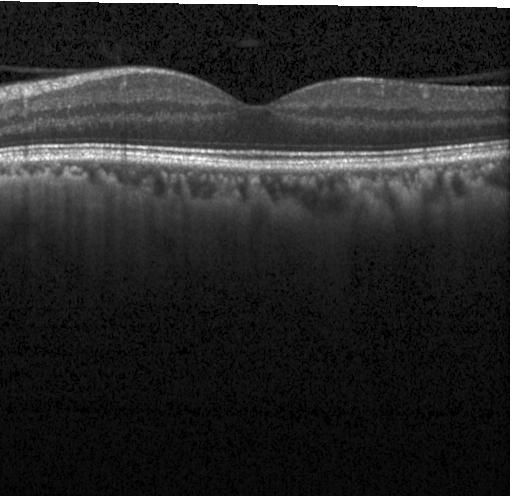 OCT line scan. Dx: no choroidal neovascularization, no diabetic macular edema, and no drusen.